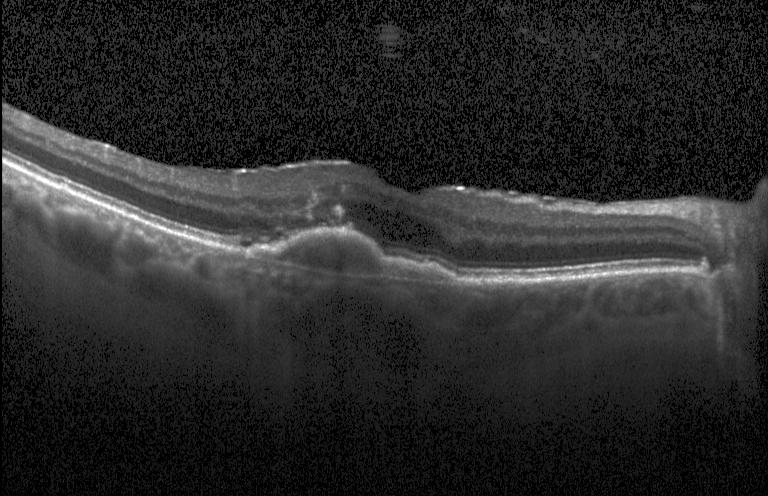 OCT B-scan — Dx: a choroidal neovascular membrane.